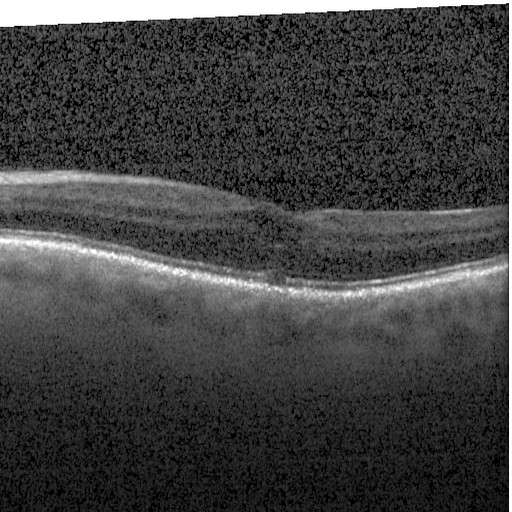 OCT B-scan — Assessment: DME.